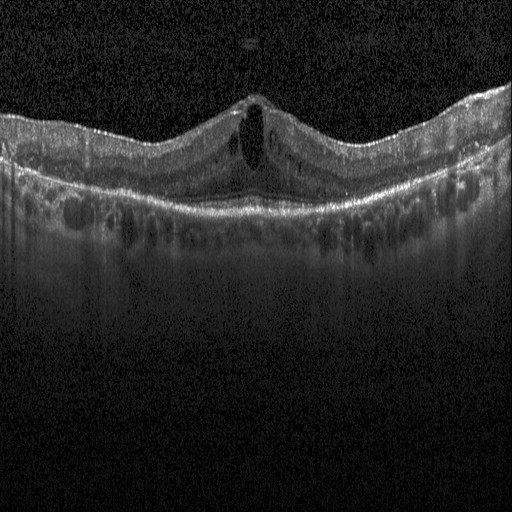
Retinal OCT cross-section showing diabetic macular edema.